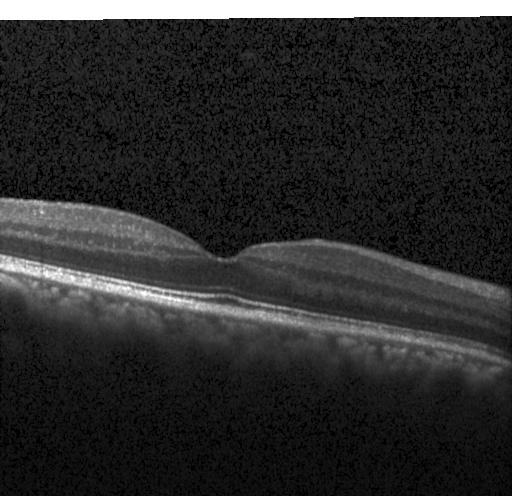 Optical coherence tomography B-scan, horizontal scan through the fovea — Finding: no choroidal neovascularization, no diabetic macular edema, and no drusen.